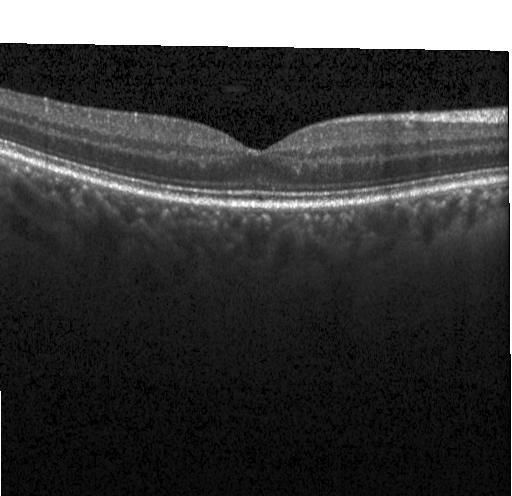 Macular OCT: no choroidal neovascularization, diabetic macular edema, or drusen.